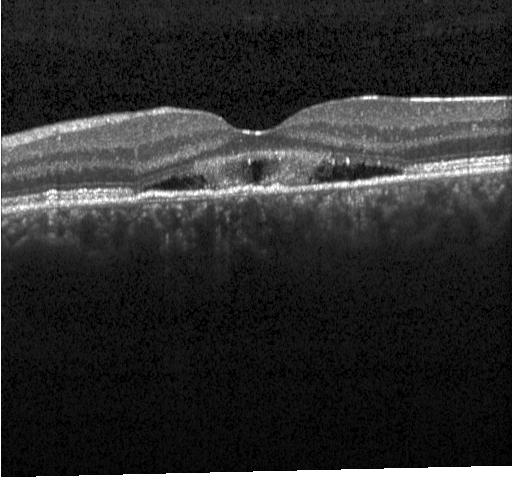
OCT finding: a choroidal neovascular membrane.